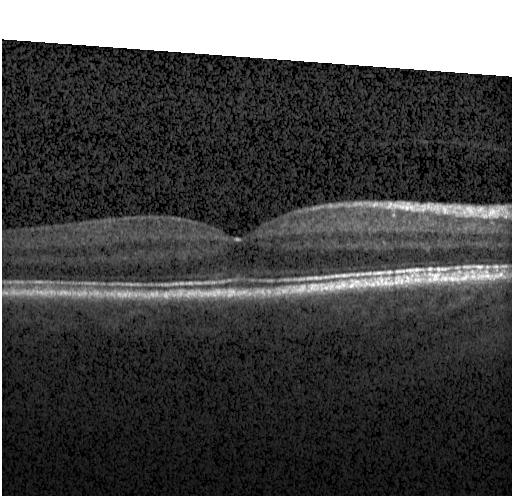 OCT scan showing no evidence of choroidal neovascularization, diabetic macular edema, or drusen.